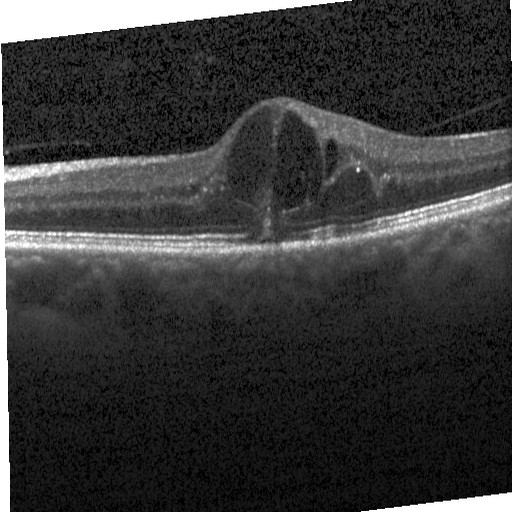

Heidelberg Spectralis · spectral-domain optical coherence tomography · optical coherence tomography B-scan.
Impression: diabetic macular edema (DME).